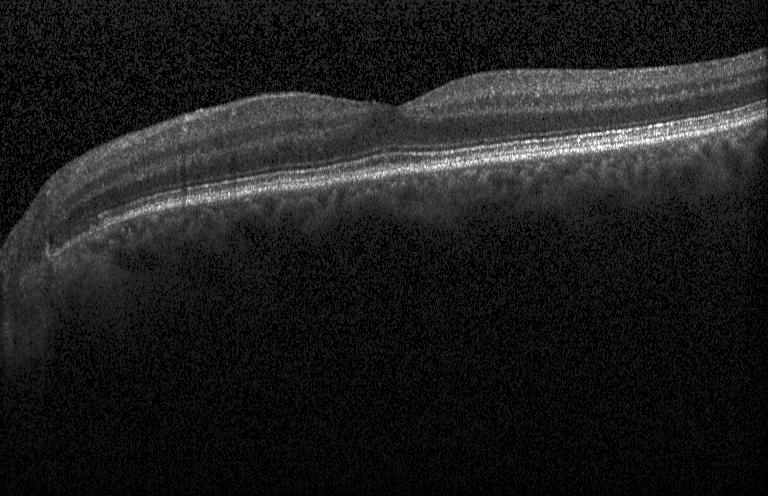 OCT line scan.
Impression: no CNV, no DME, and no drusen.